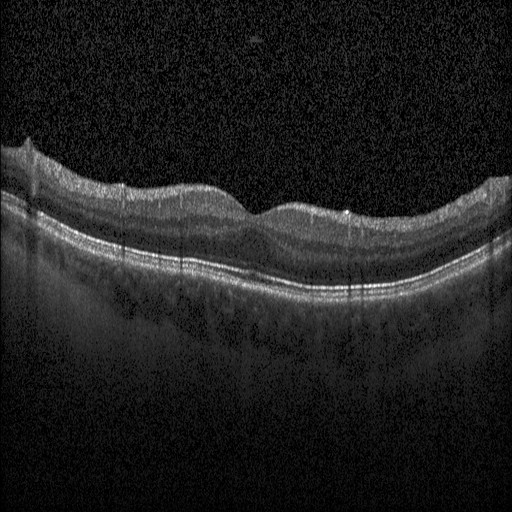
Instrument: Heidelberg Spectralis · through the macula · OCT B-scan.
This B-scan demonstrates diabetic macular edema.